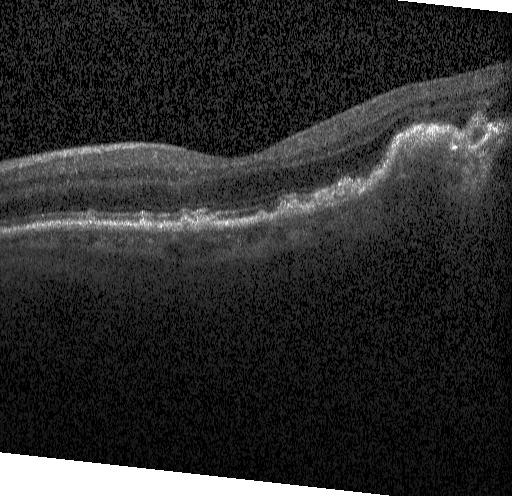 Macular OCT demonstrating choroidal neovascularization (CNV).